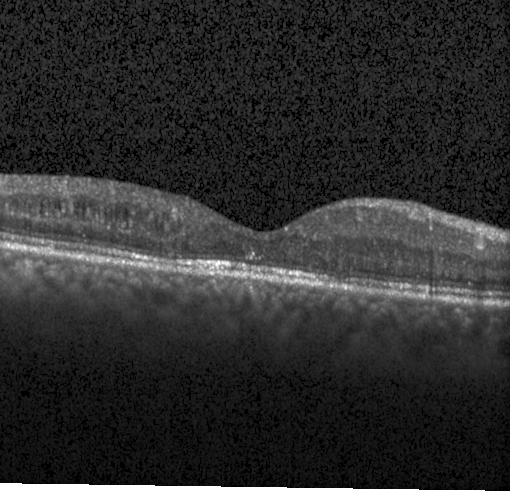

Spectral-domain OCT, OCT B-scan — The scan shows DME.